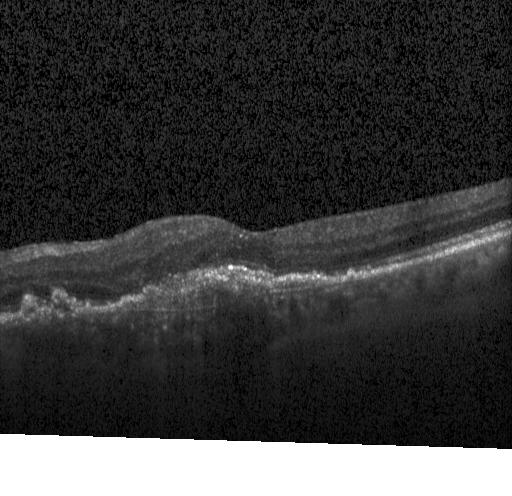

OCT line scan · fovea-centered · instrument: Heidelberg Spectralis · SD-OCT. Finding: a choroidal neovascular membrane.